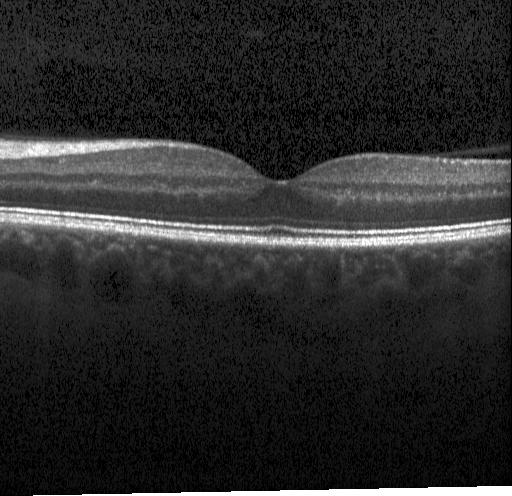 Acquired on a Heidelberg Spectralis, retinal OCT B-scan, macular scan.
Finding: no evidence of choroidal neovascularization, diabetic macular edema, or drusen.